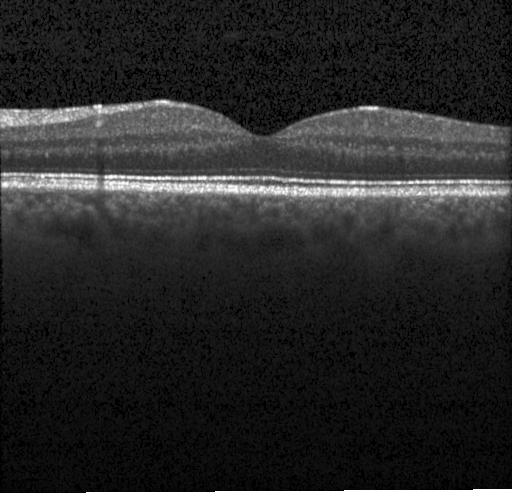

Retinal OCT cross-section · fovea-centered — Diagnosis: neither CNV, DME, nor drusen.